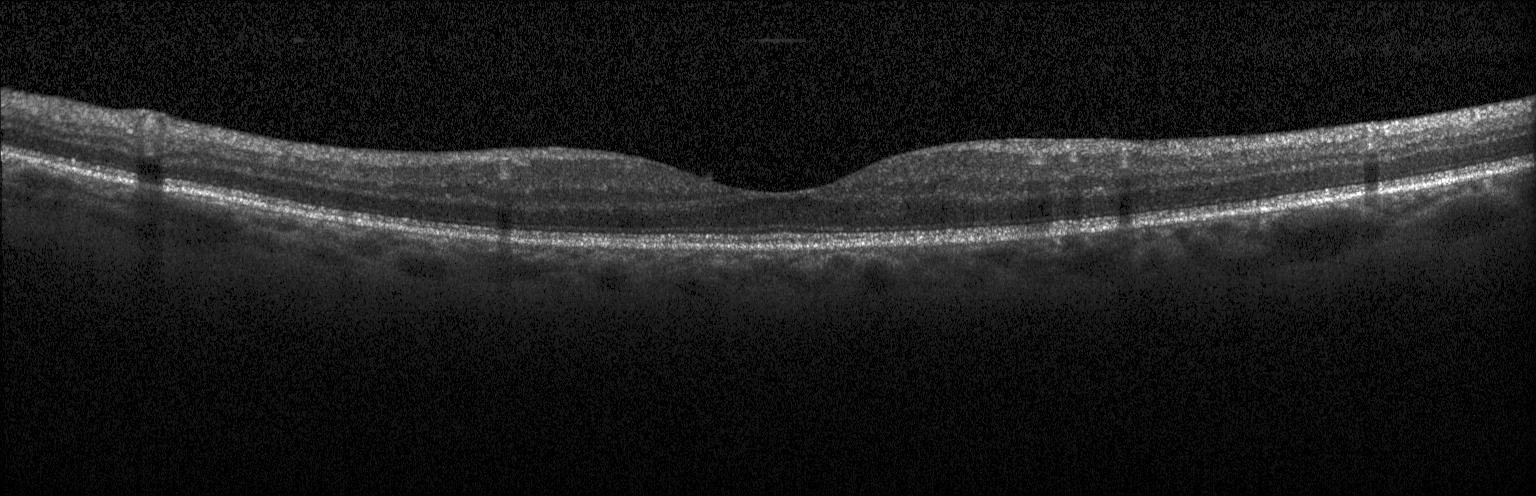

Retinal OCT cross-section. Through the macula. Instrument: Heidelberg Spectralis. Spectral-domain optical coherence tomography.
No choroidal neovascularization, diabetic macular edema, or drusen.